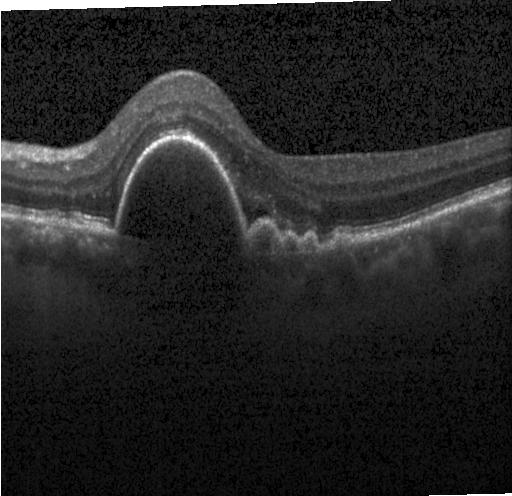 A choroidal neovascular membrane.